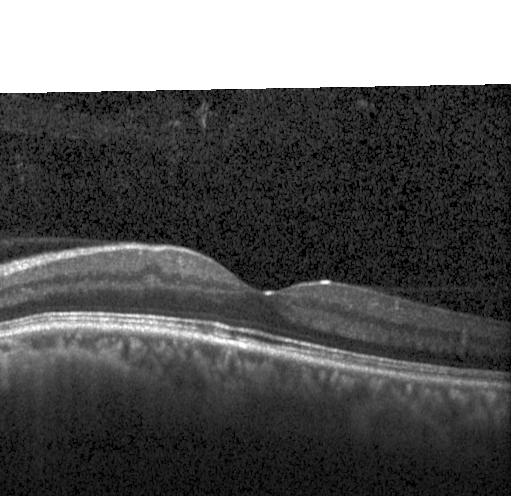 Optical coherence tomography scan · Heidelberg Spectralis · spectral-domain optical coherence tomography — No choroidal neovascularization, no diabetic macular edema, and no drusen.